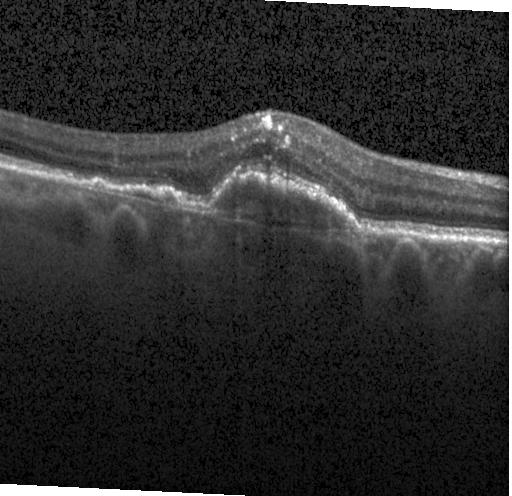
OCT B-scan showing choroidal neovascularization.